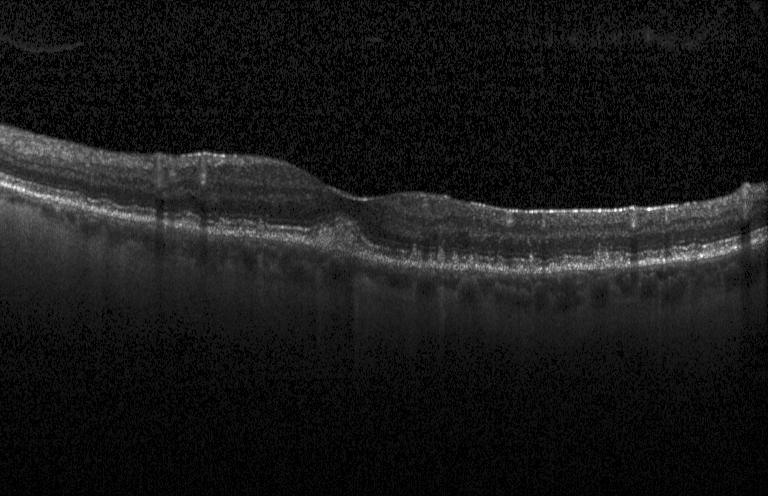 Diagnosis: sub-RPE drusenoid deposits.